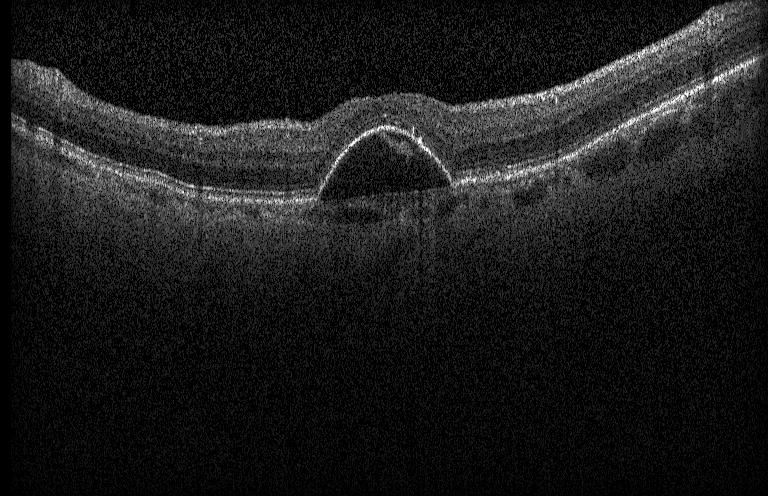

Retinal OCT B-scan — CNV.